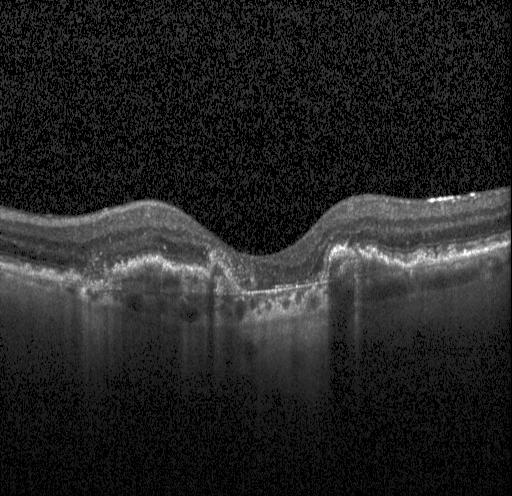 Finding: a choroidal neovascular membrane.